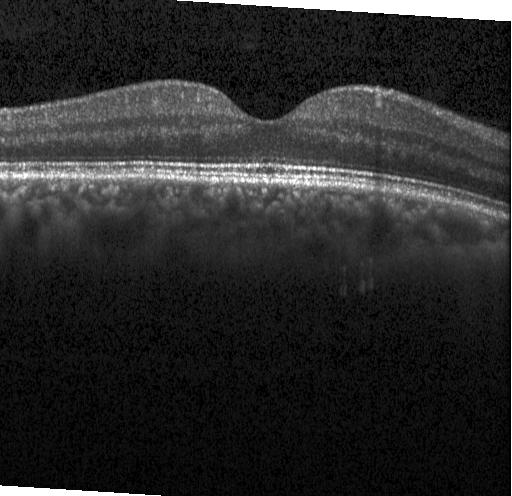
Macular OCT demonstrating no evidence of CNV, DME, or drusen.